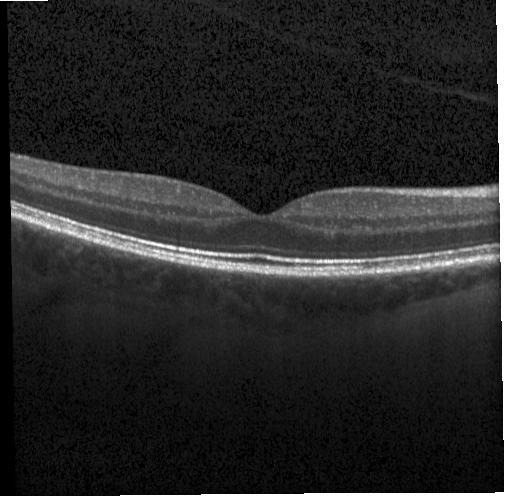
Macular OCT: no choroidal neovascularization, diabetic macular edema, or drusen.